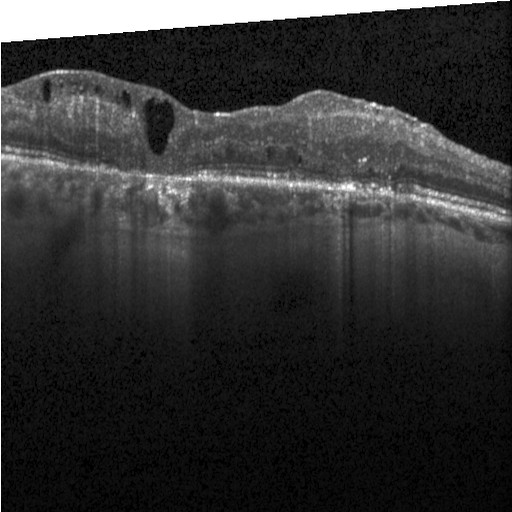

OCT line scan. SD-OCT. OCT finding: diabetic macular edema.